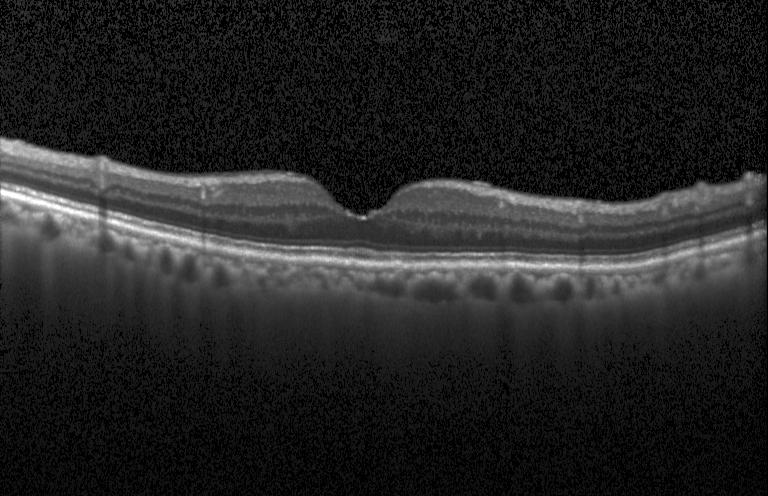
Retinal OCT B-scan · spectral-domain OCT · centered on the fovea.
Impression: neither CNV, DME, nor drusen.